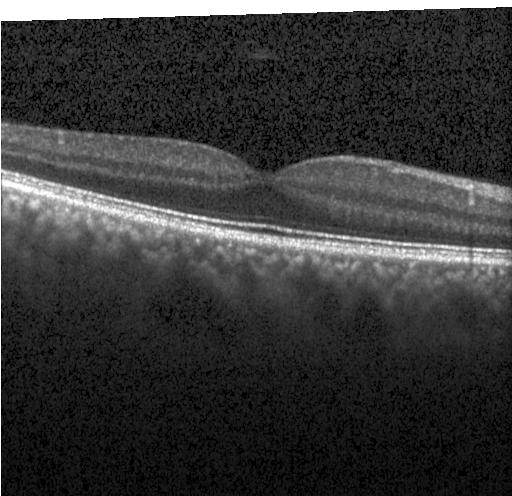

Spectral-domain OCT. Instrument: Heidelberg Spectralis. Centered on the fovea. Optical coherence tomography scan.
Assessment: neither CNV, DME, nor drusen.